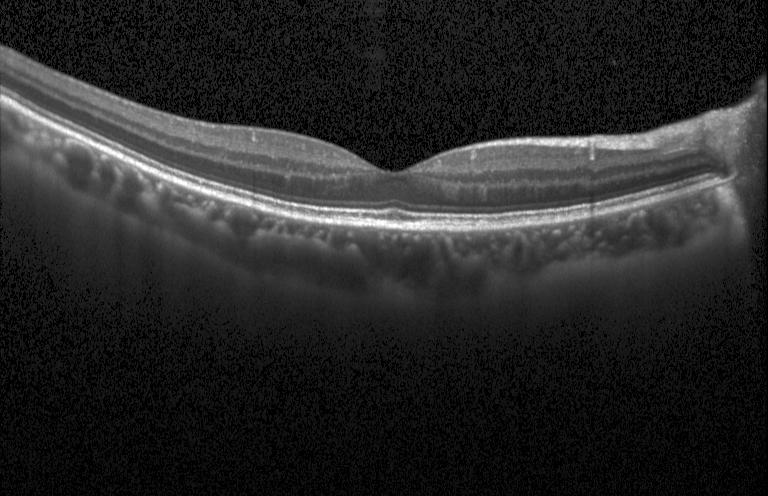

This B-scan demonstrates no choroidal neovascularization, no diabetic macular edema, and no drusen.